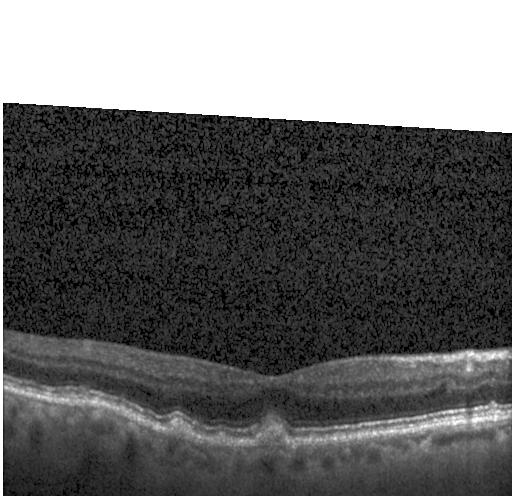 SD-OCT · OCT line scan. This B-scan demonstrates sub-RPE drusenoid deposits.